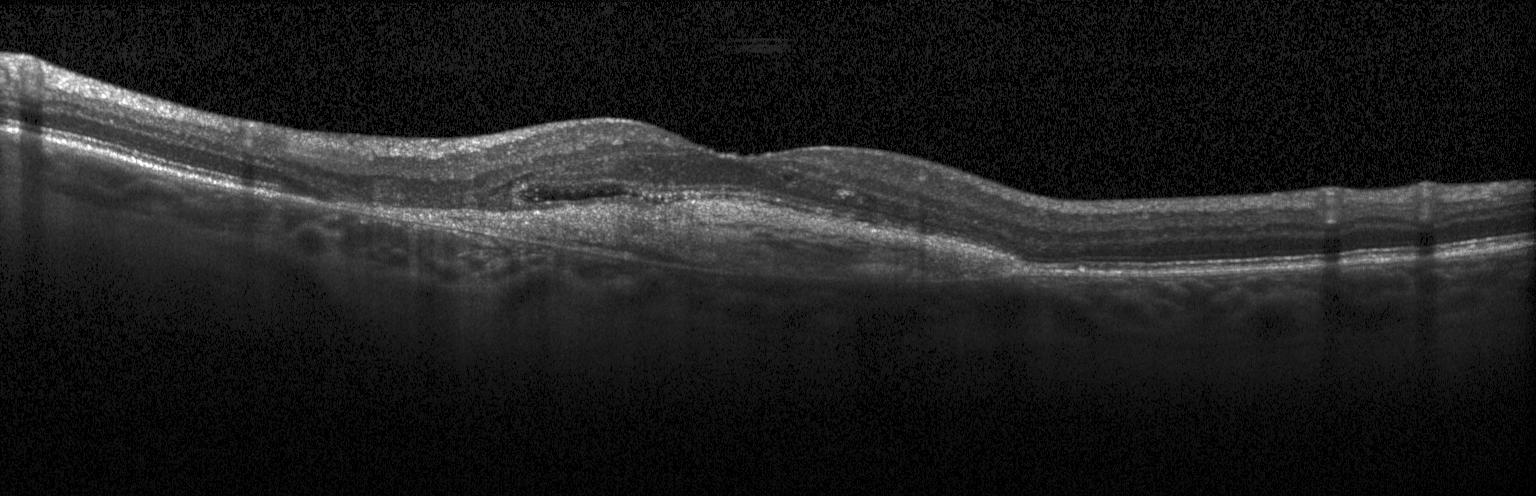 This B-scan demonstrates choroidal neovascularization.